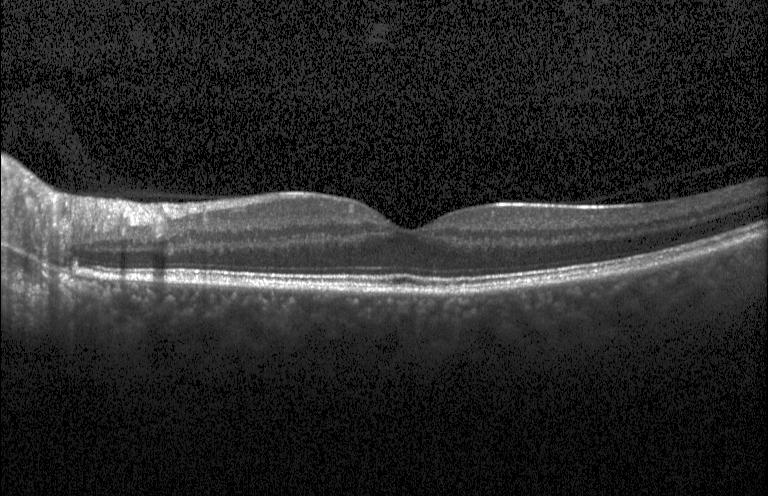 Optical coherence tomography scan. Heidelberg Spectralis
Impression: no evidence of choroidal neovascularization, diabetic macular edema, or drusen.